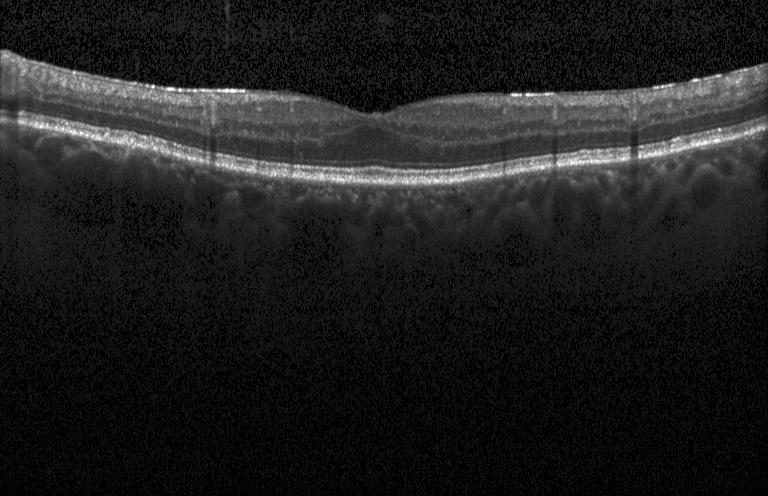 Retinal OCT B-scan. Instrument: Heidelberg Spectralis. Macular scan.
The scan shows neither CNV, DME, nor drusen.